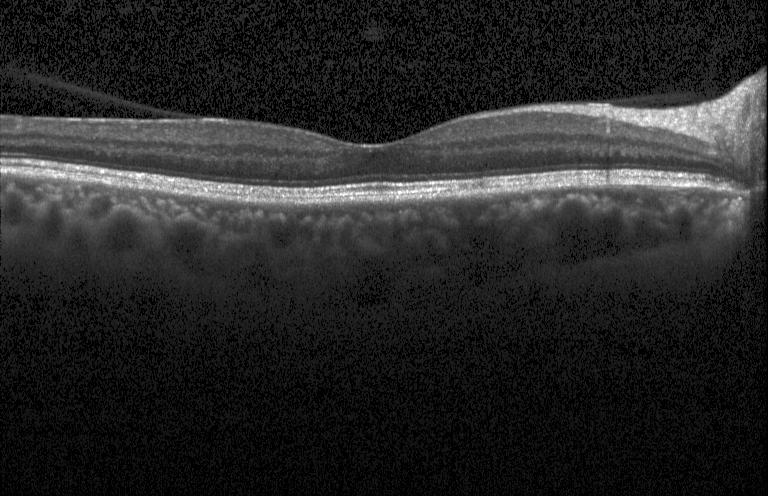
Heidelberg Spectralis OCT system. Retinal OCT B-scan. SD-OCT. Macular scan — Diagnosis: no evidence of choroidal neovascularization, diabetic macular edema, or drusen.